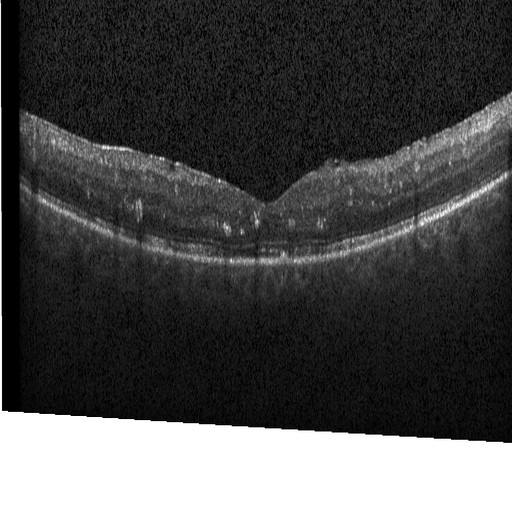 OCT scan showing diabetic macular edema.